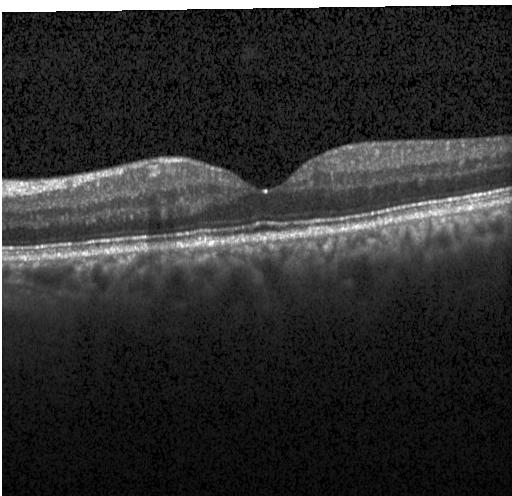
Retinal OCT B-scan; Heidelberg Spectralis OCT system; through the macula.
This B-scan demonstrates no choroidal neovascularization, diabetic macular edema, or drusen.